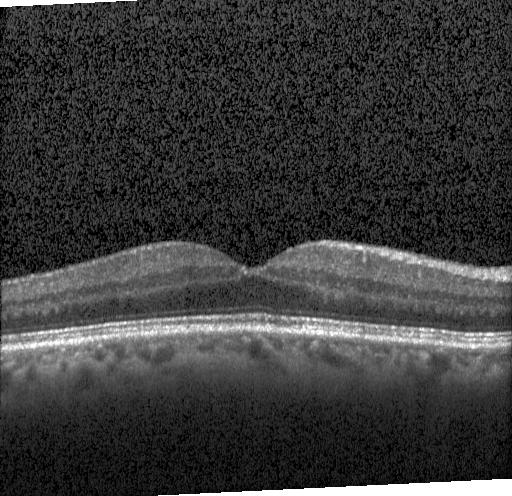 The scan shows neither choroidal neovascularization, diabetic macular edema, nor drusen.